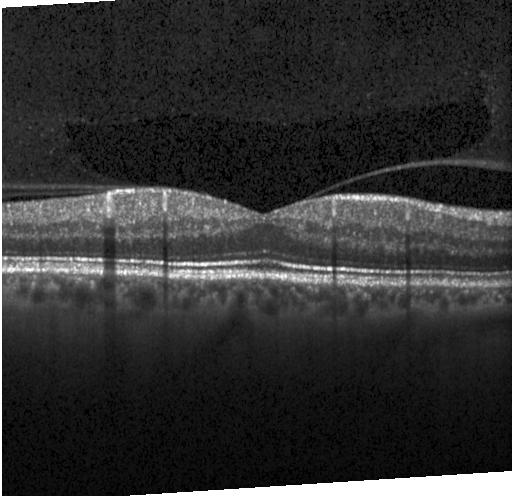

SD-OCT · OCT B-scan.
Neither choroidal neovascularization, diabetic macular edema, nor drusen.